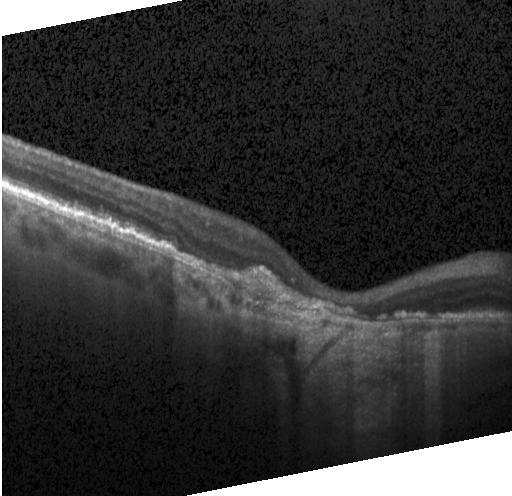
Instrument: Heidelberg Spectralis, optical coherence tomography scan
Assessment: a choroidal neovascular membrane.